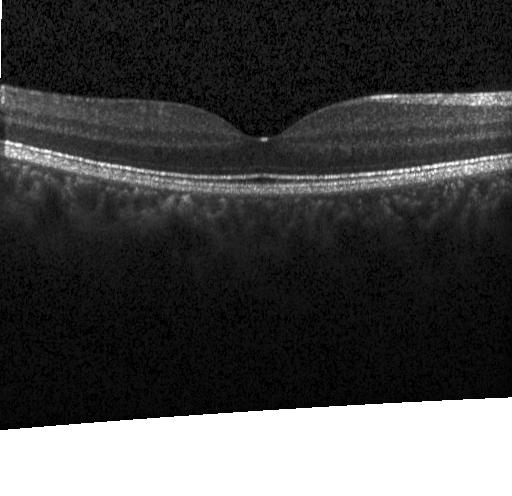 Retinal OCT cross-section · spectral-domain OCT · acquired on a Heidelberg Spectralis · through the macula. Diagnosis: neither choroidal neovascularization, diabetic macular edema, nor drusen.